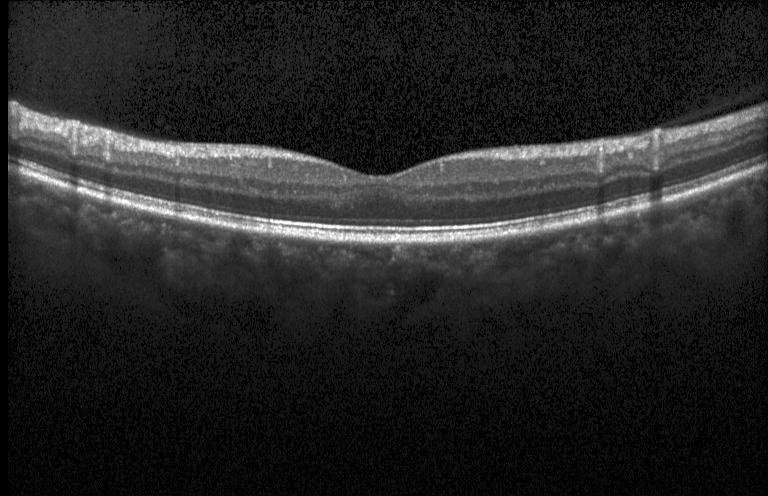 Instrument: Heidelberg Spectralis; retinal OCT B-scan; spectral-domain optical coherence tomography.
Macular OCT: no choroidal neovascularization, diabetic macular edema, or drusen.